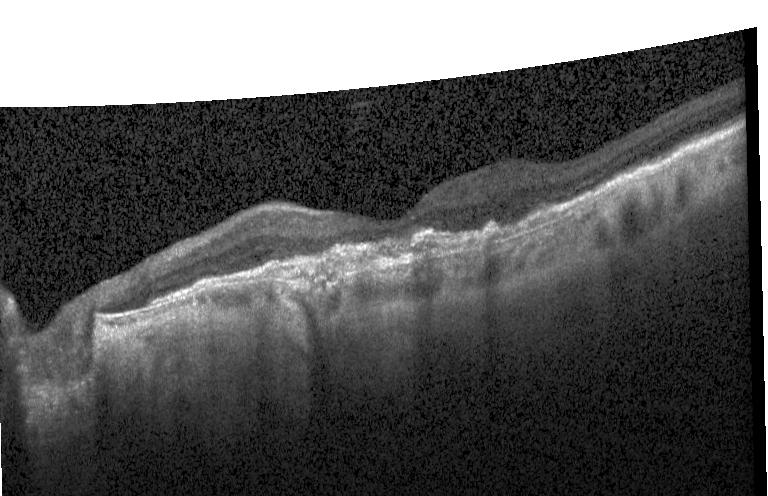 Optical coherence tomography B-scan — Impression: CNV.